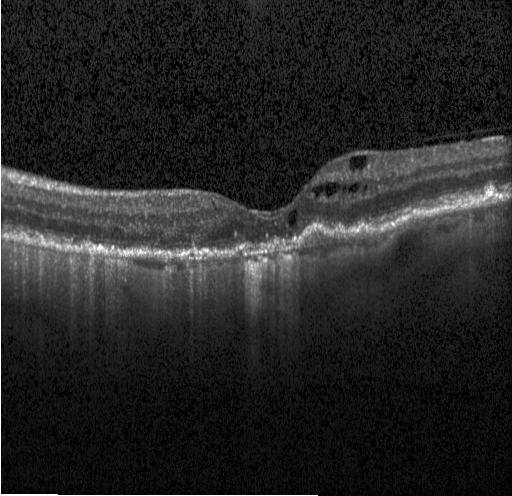

Macular scan. OCT B-scan. SD-OCT. Impression: choroidal neovascularization (CNV).